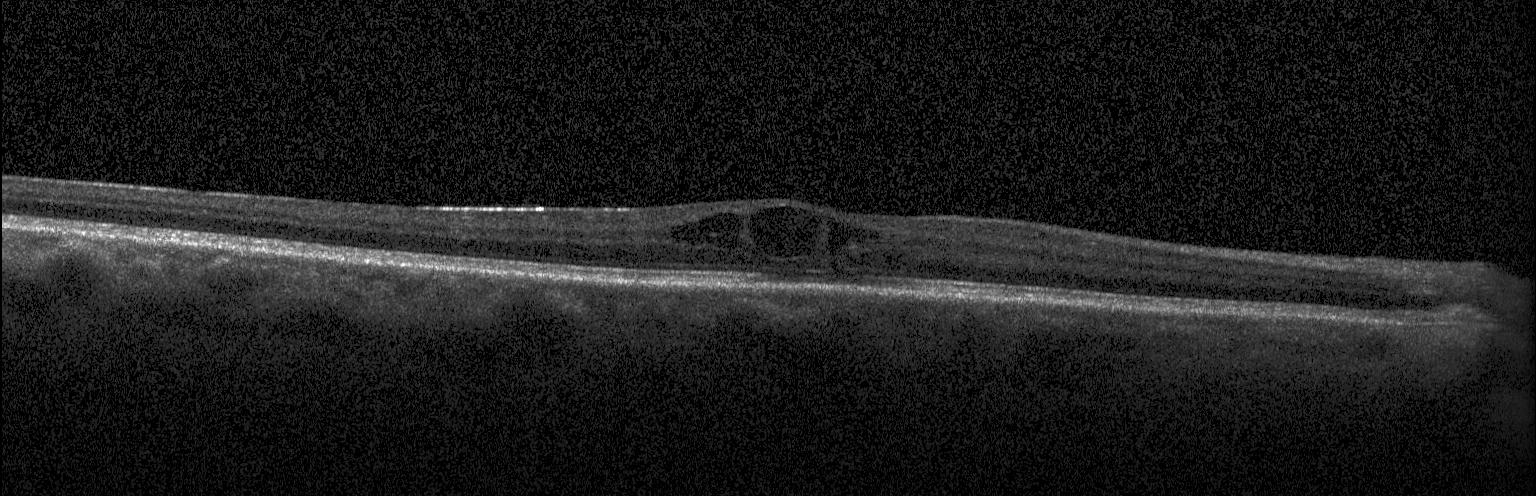

SD-OCT. Acquired on a Heidelberg Spectralis. Macular scan. OCT line scan. Diabetic macular edema (DME).